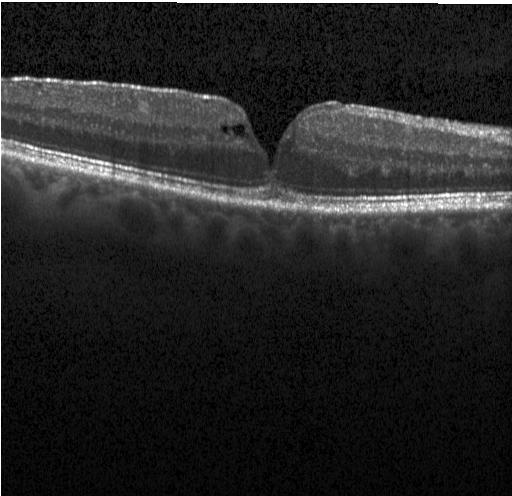
OCT line scan — Diagnosis: diabetic macular edema (DME).